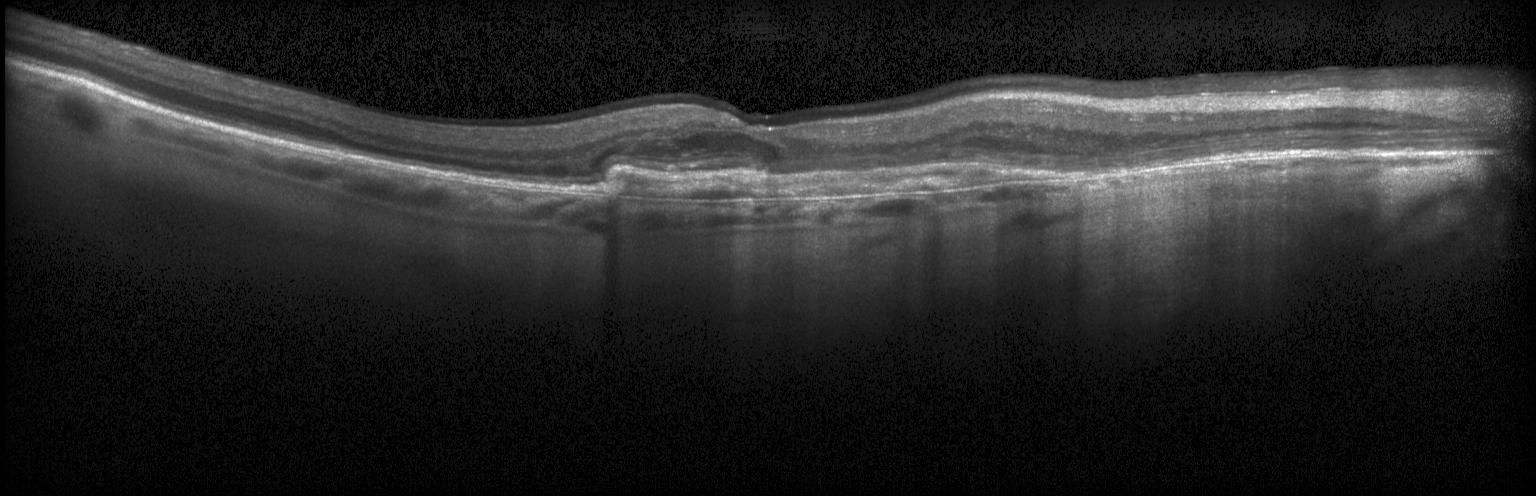
Assessment: a choroidal neovascular membrane.